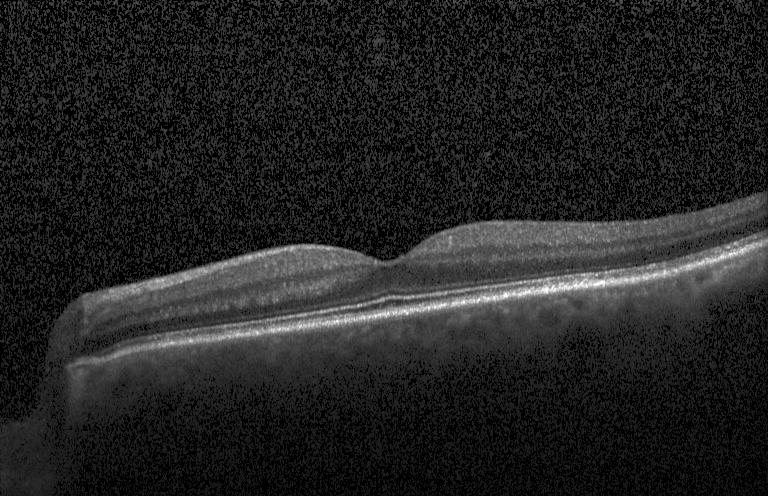
Impression: no CNV, no DME, and no drusen.